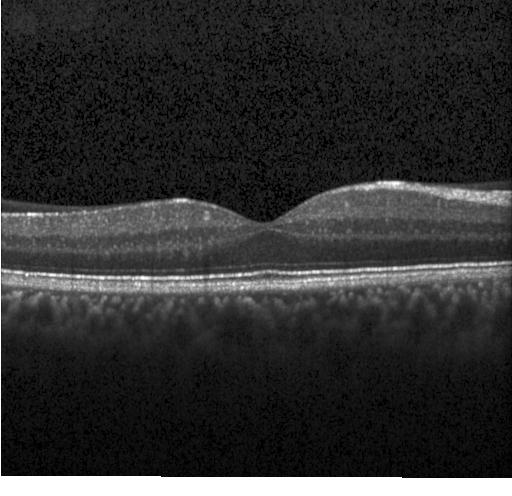

Retinal OCT B-scan
Assessment: no evidence of CNV, DME, or drusen.